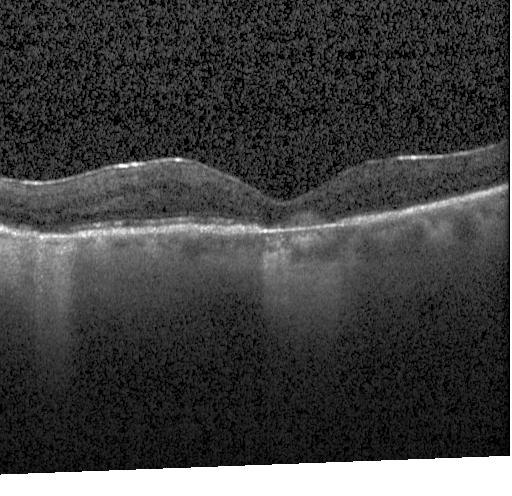 Instrument: Heidelberg Spectralis · through the macula · optical coherence tomography scan · SD-OCT. A choroidal neovascular membrane.